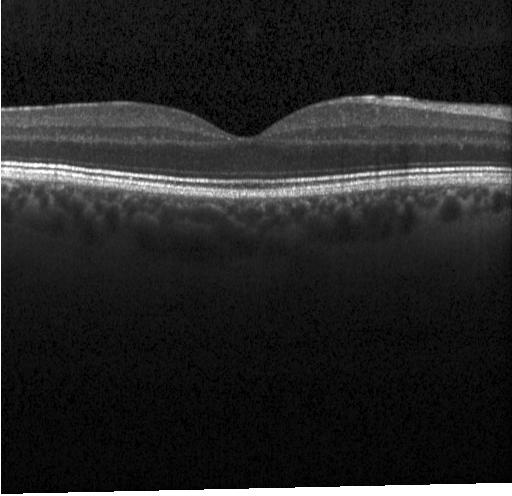

OCT scan showing neither choroidal neovascularization, diabetic macular edema, nor drusen.